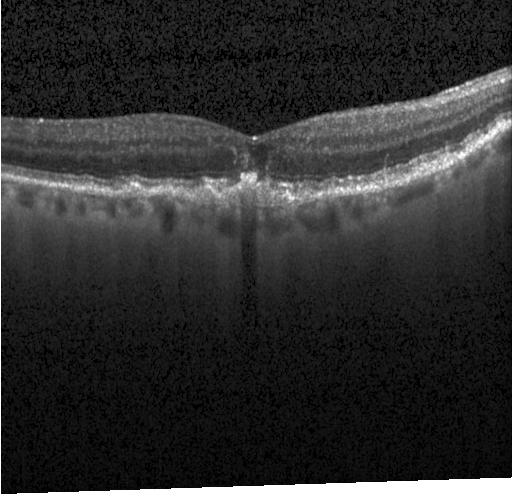

Dx: a choroidal neovascular membrane.